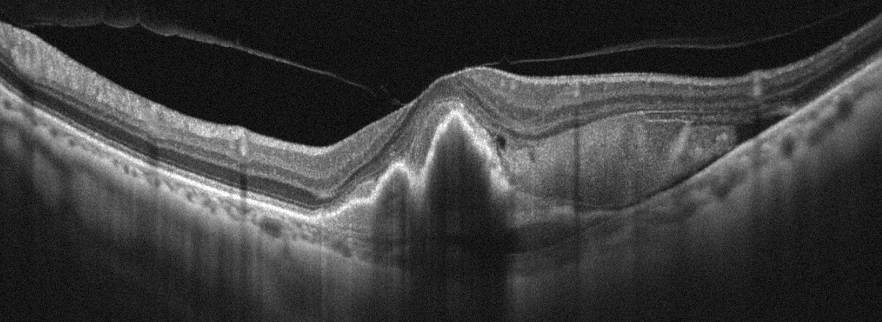
Finding: age-related macular degeneration.